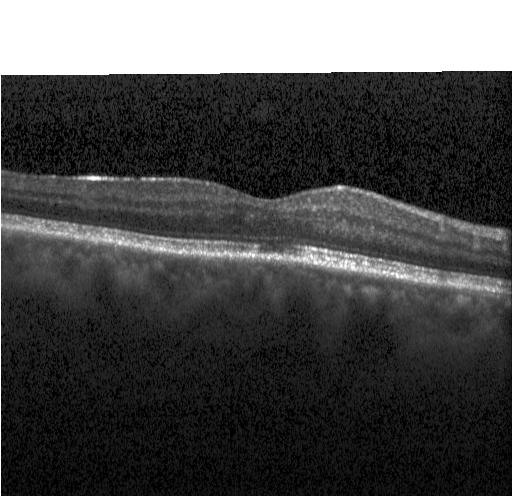 Macular scan · retinal OCT B-scan · spectral-domain optical coherence tomography.
Diagnosis: neither choroidal neovascularization, diabetic macular edema, nor drusen.